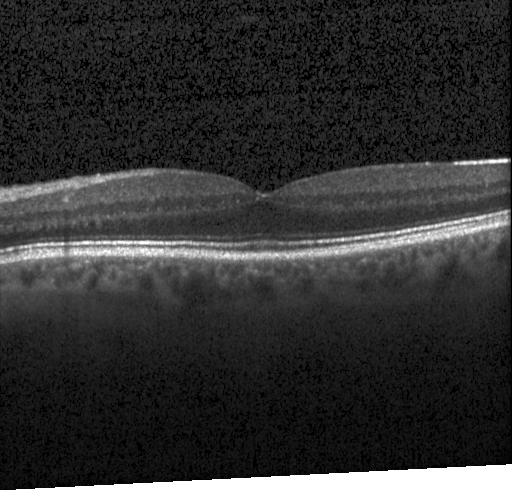 Retinal OCT B-scan · spectral-domain optical coherence tomography · acquired on a Heidelberg Spectralis — OCT finding: no choroidal neovascularization, diabetic macular edema, or drusen.